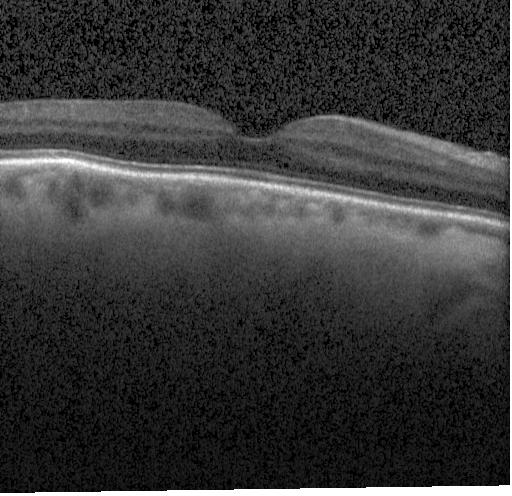

SD-OCT. Retinal OCT cross-section. Heidelberg Spectralis.
This B-scan demonstrates no evidence of CNV, DME, or drusen.